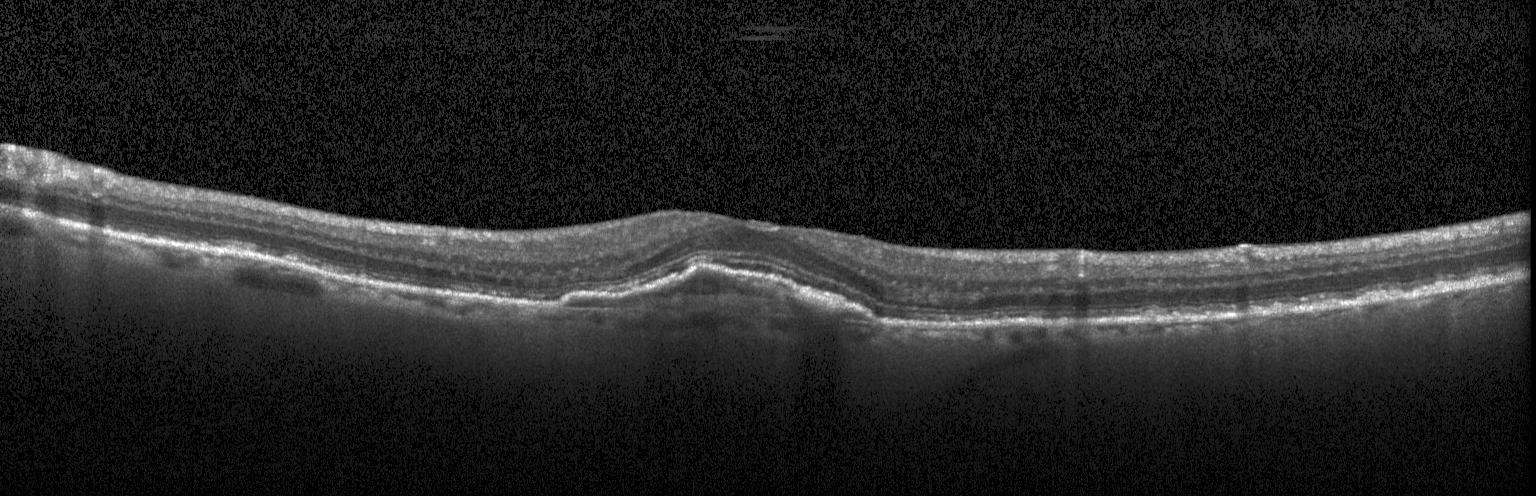 Optical coherence tomography B-scan. Macular OCT: CNV.